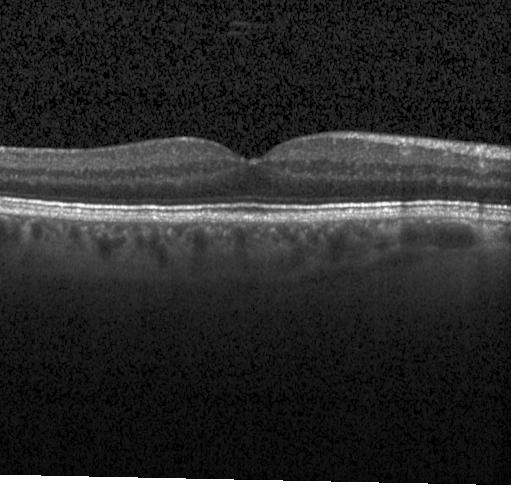
Optical coherence tomography B-scan
Dx: no choroidal neovascularization, diabetic macular edema, or drusen.